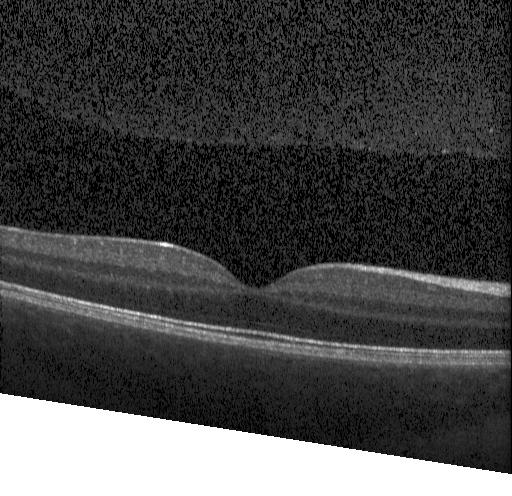
Fovea-centered, optical coherence tomography scan, spectral-domain optical coherence tomography.
Dx: neither choroidal neovascularization, diabetic macular edema, nor drusen.